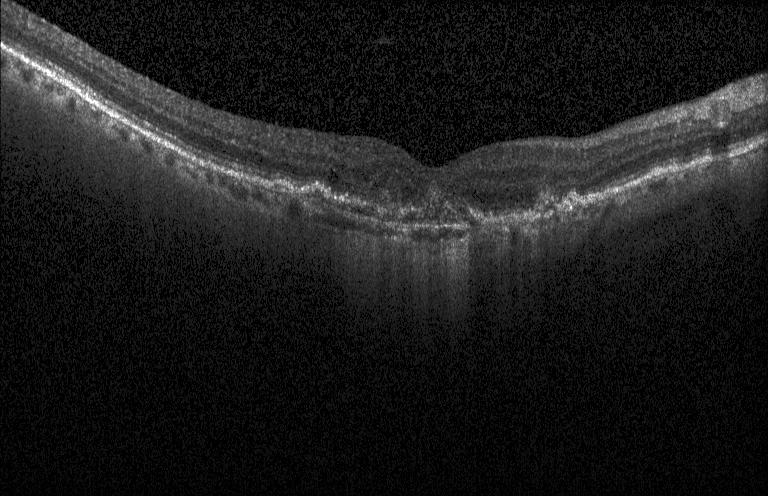 Retinal OCT B-scan. Horizontal scan through the fovea. Spectral-domain optical coherence tomography
A choroidal neovascular membrane.